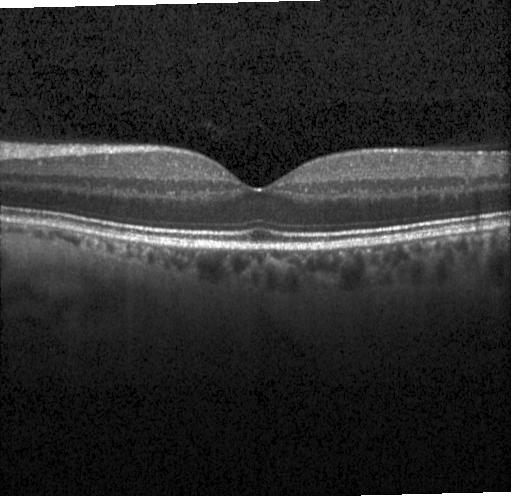

Retinal OCT cross-section — The scan shows no choroidal neovascularization, no diabetic macular edema, and no drusen.